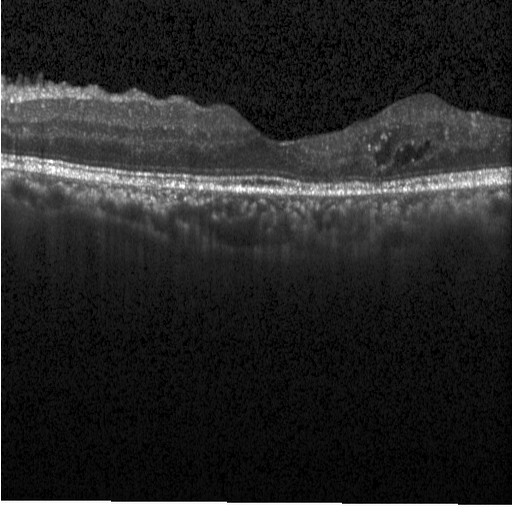
Spectral-domain optical coherence tomography, retinal OCT B-scan, horizontal scan through the fovea, Heidelberg Spectralis OCT system.
The scan shows diabetic macular edema.